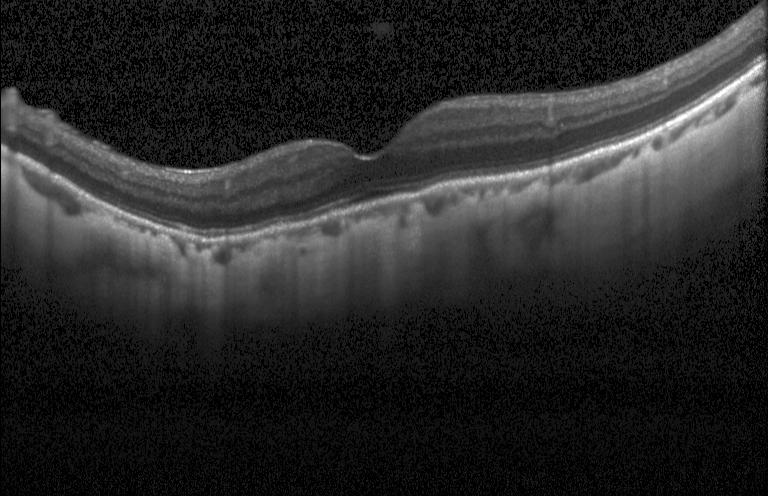

This B-scan demonstrates neither choroidal neovascularization, diabetic macular edema, nor drusen.